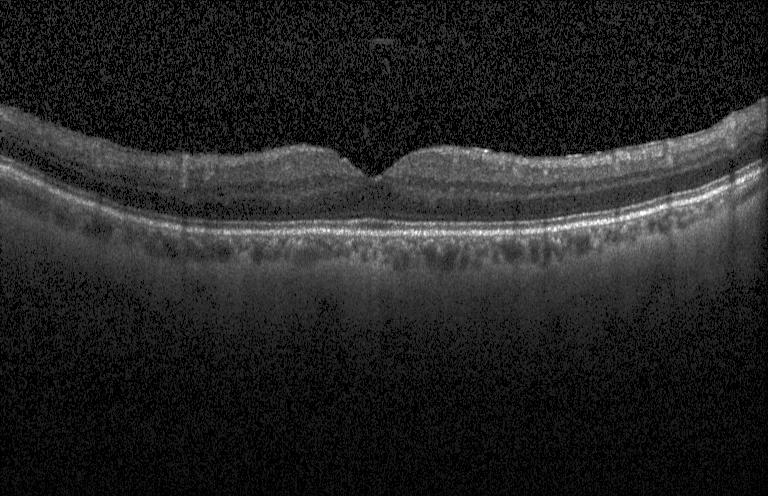
Optical coherence tomography B-scan; SD-OCT; through the macula — Impression: no CNV, DME, or drusen.